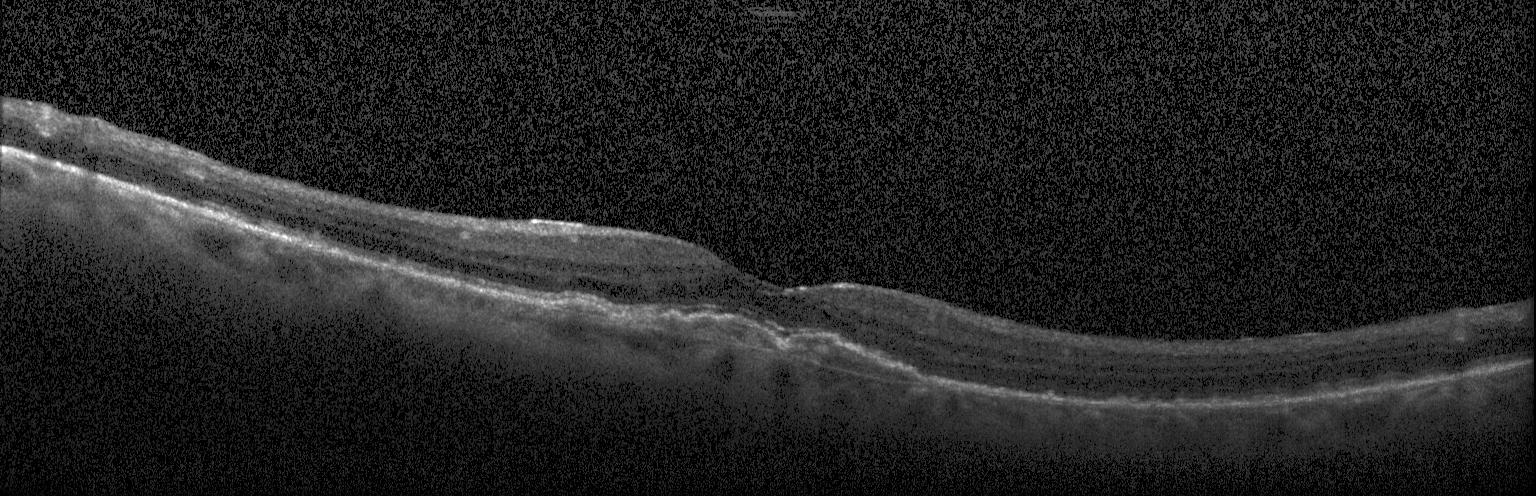 Retinal OCT B-scan. Macular OCT: CNV.